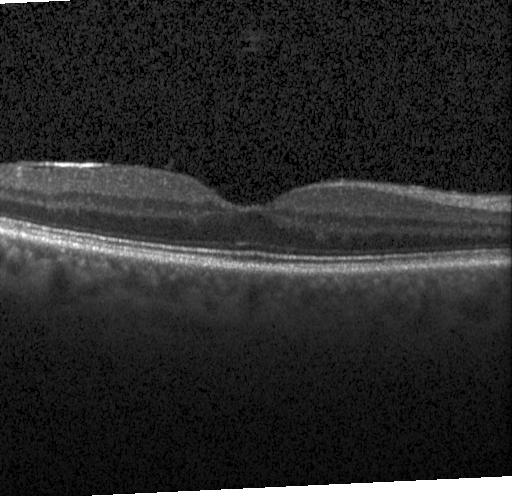
Retinal OCT B-scan — Finding: no choroidal neovascularization, diabetic macular edema, or drusen.